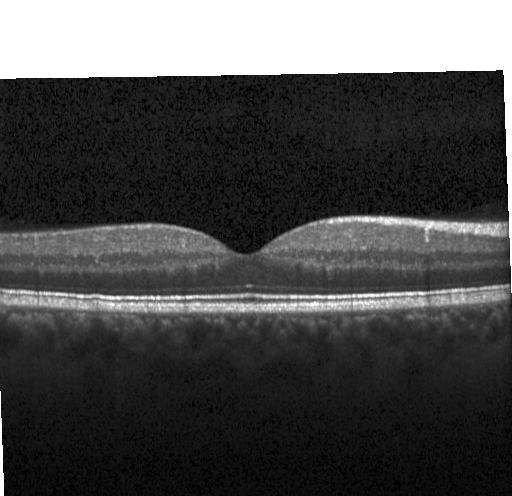
Spectral-domain OCT B-scan: no choroidal neovascularization, no diabetic macular edema, and no drusen.